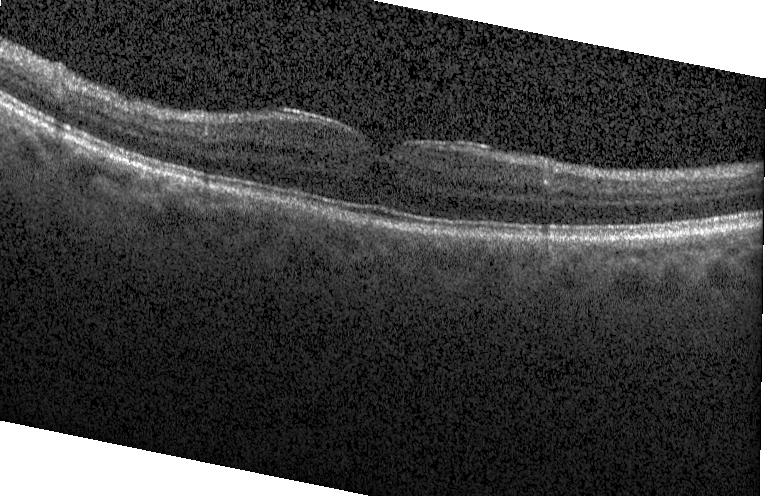
Finding: no choroidal neovascularization, diabetic macular edema, or drusen.